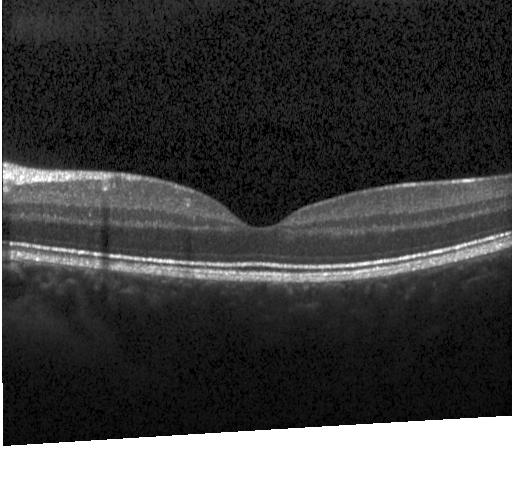

OCT B-scan showing no evidence of choroidal neovascularization, diabetic macular edema, or drusen.